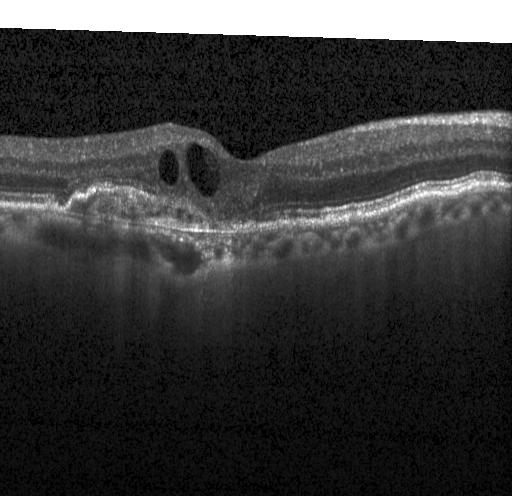
Optical coherence tomography scan
The scan shows choroidal neovascularization.